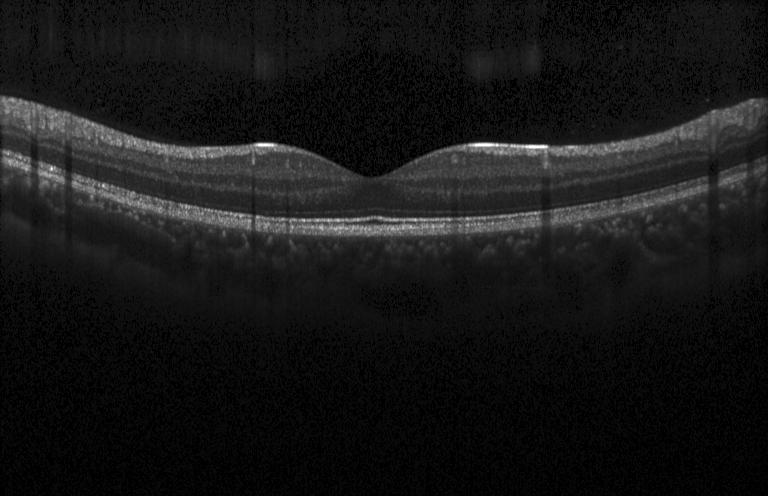

Retinal OCT cross-section; Heidelberg Spectralis — OCT finding: no choroidal neovascularization, diabetic macular edema, or drusen.